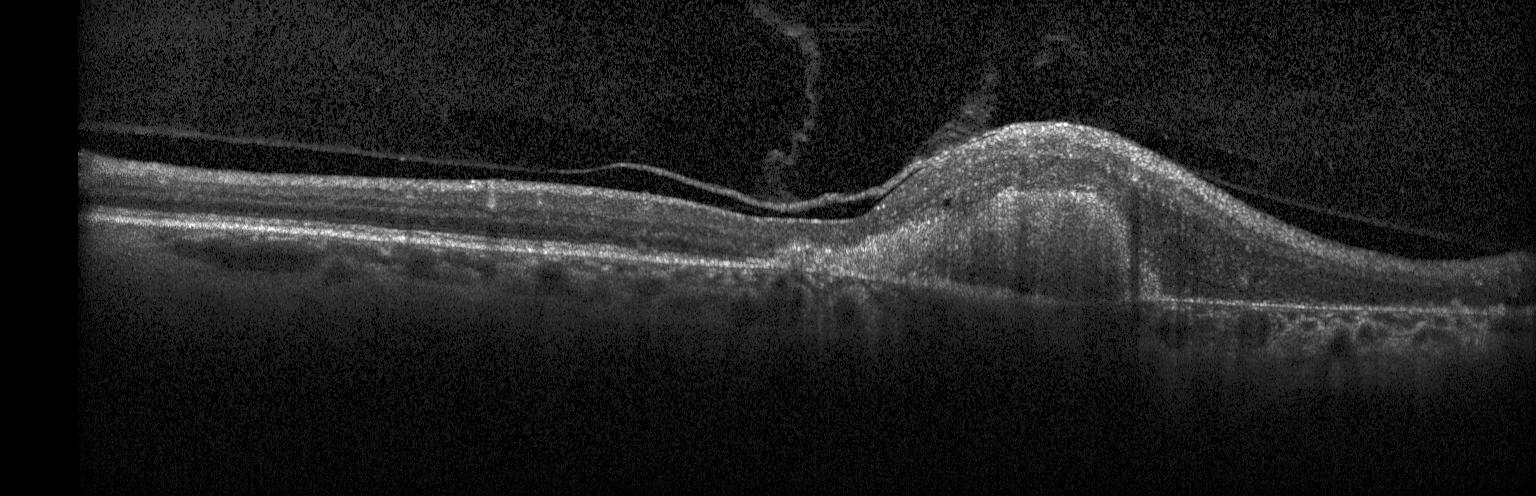

Through the macula, optical coherence tomography scan, SD-OCT. Finding: choroidal neovascularization (CNV).